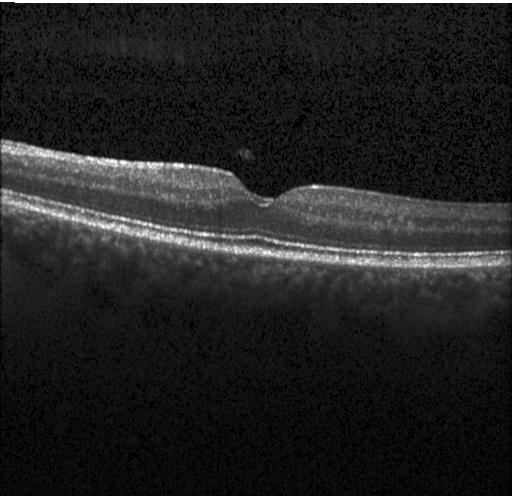

Diagnosis: no evidence of choroidal neovascularization, diabetic macular edema, or drusen.